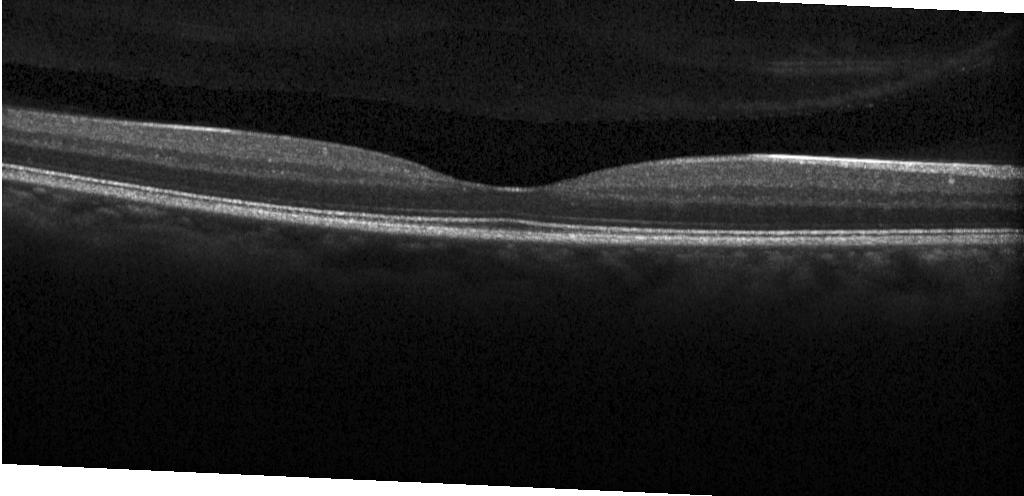
OCT B-scan. Assessment: no CNV, no DME, and no drusen.